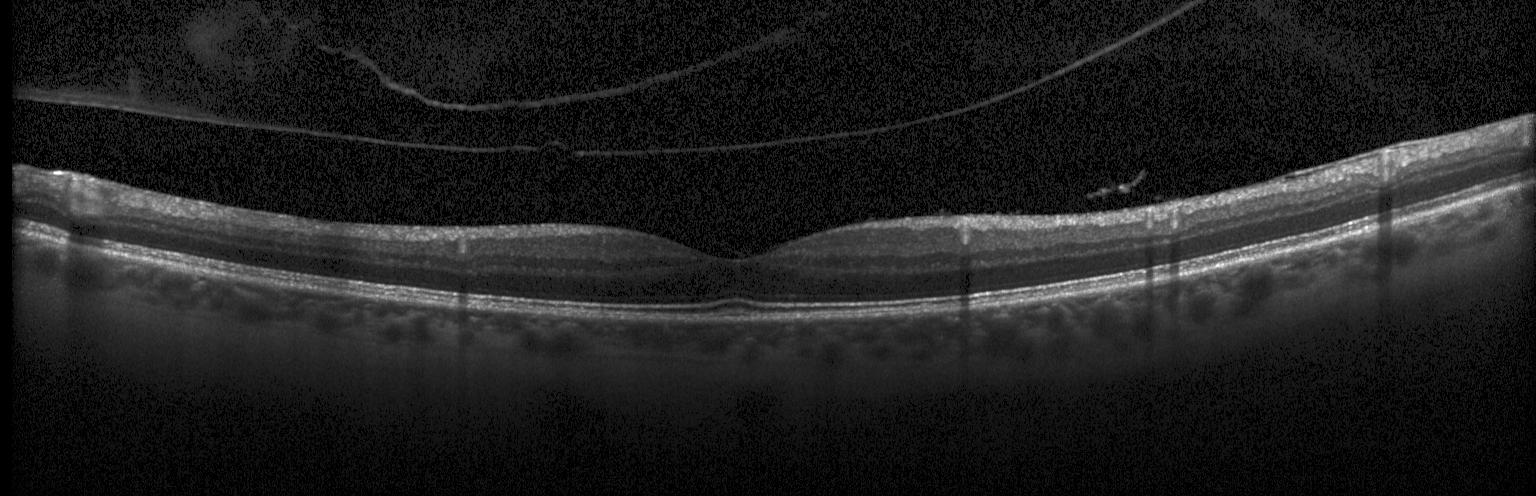

No choroidal neovascularization, no diabetic macular edema, and no drusen.